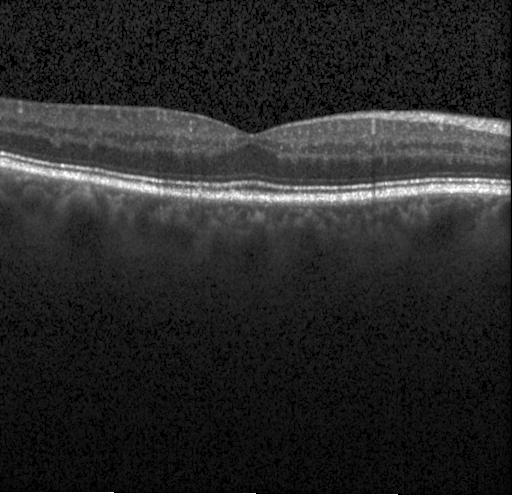

Optical coherence tomography B-scan, Heidelberg Spectralis OCT system — Macular OCT: no choroidal neovascularization, diabetic macular edema, or drusen.